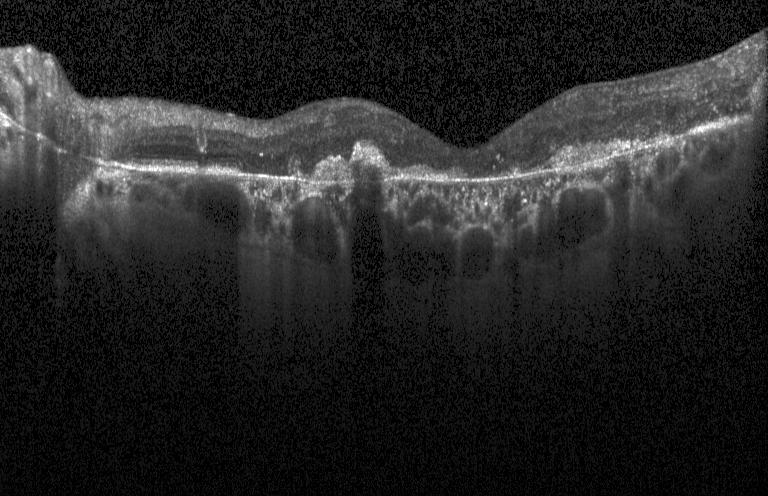
Diagnosis: a choroidal neovascular membrane.